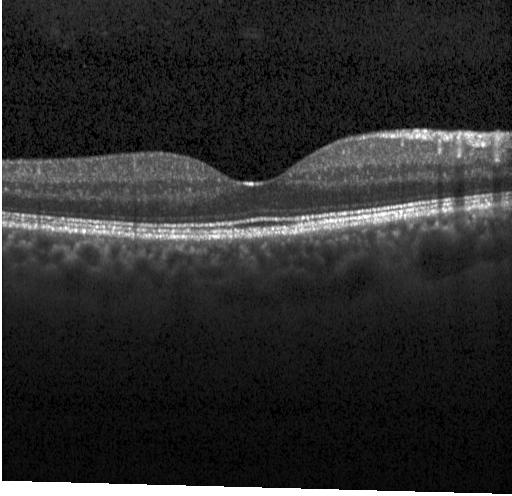

OCT scan showing no choroidal neovascularization, no diabetic macular edema, and no drusen.